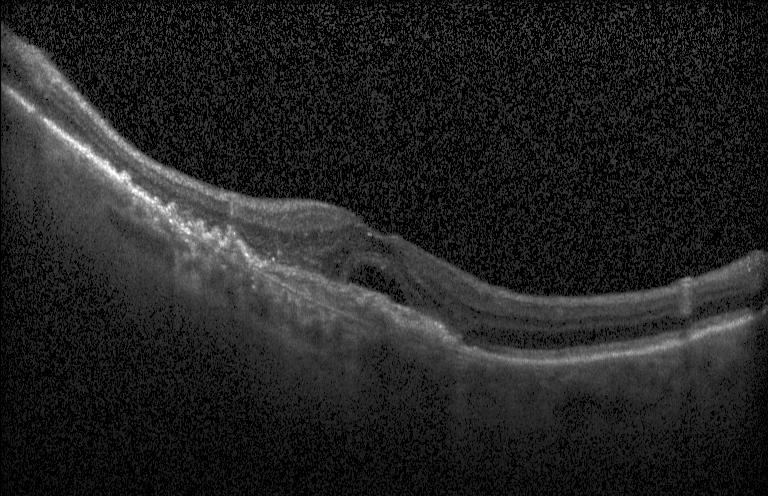

Macular OCT: choroidal neovascularization.